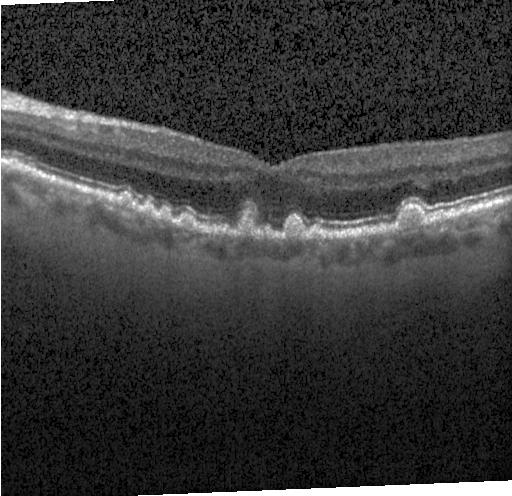 OCT B-scan; spectral-domain OCT; centered on the fovea.
OCT finding: drusen.